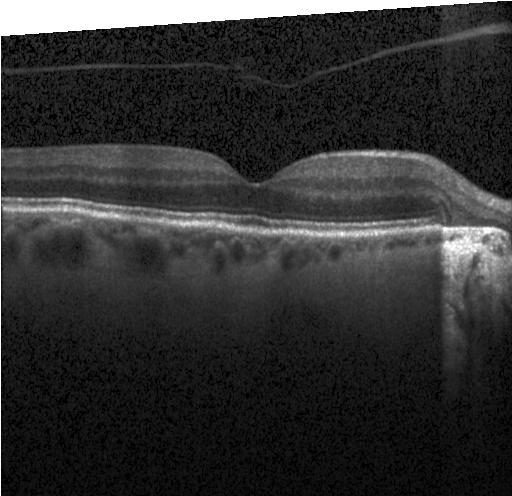

Macular OCT: no CNV, DME, or drusen.